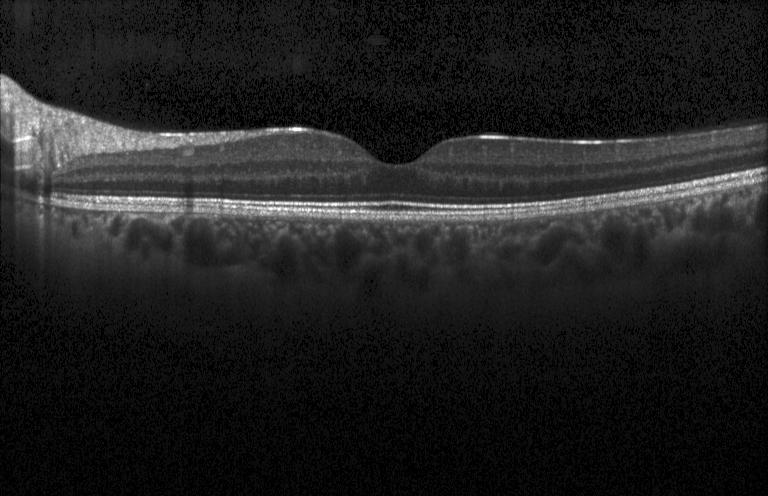
Retinal OCT cross-section — The scan shows no CNV, no DME, and no drusen.